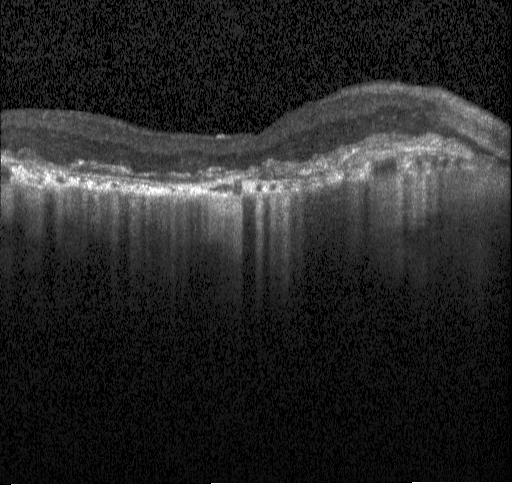 Acquired on a Heidelberg Spectralis. SD-OCT. Optical coherence tomography scan. Fovea-centered. This B-scan demonstrates choroidal neovascularization.